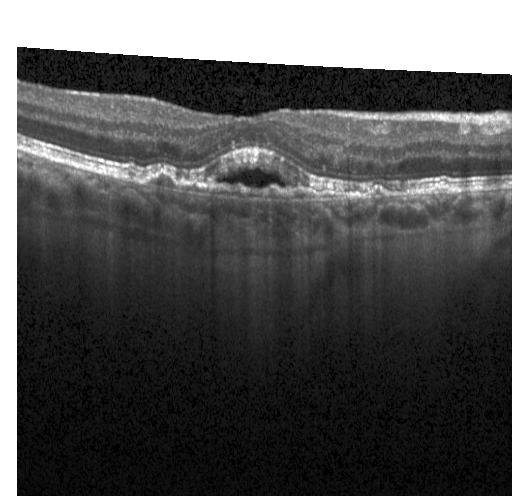

Heidelberg Spectralis OCT system. Optical coherence tomography scan. Finding: choroidal neovascularization.